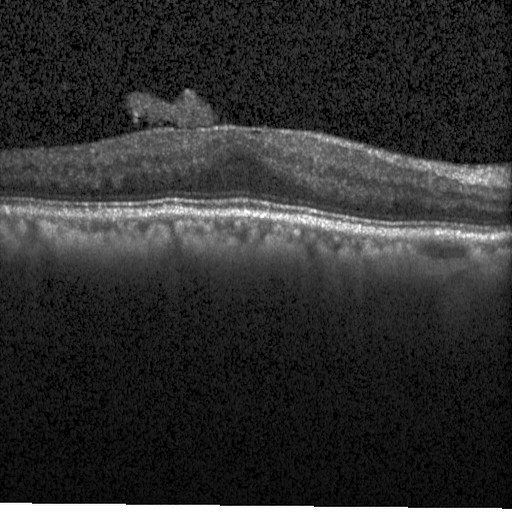

The scan shows DME.